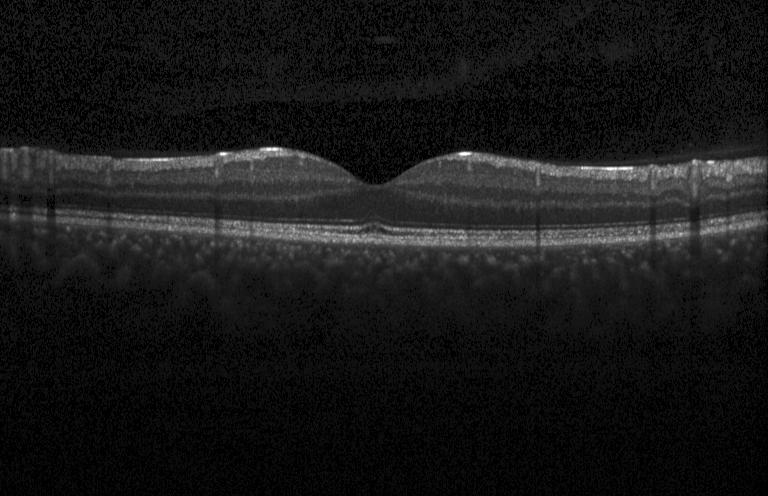

Diagnosis: neither choroidal neovascularization, diabetic macular edema, nor drusen.